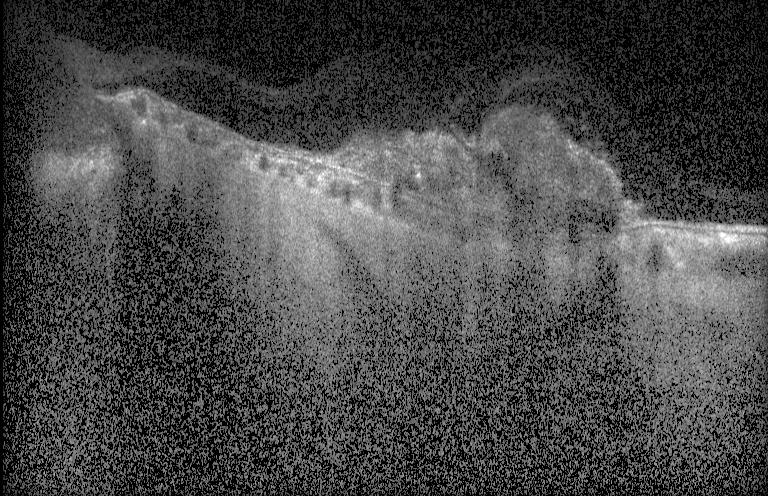 Impression: choroidal neovascularization.